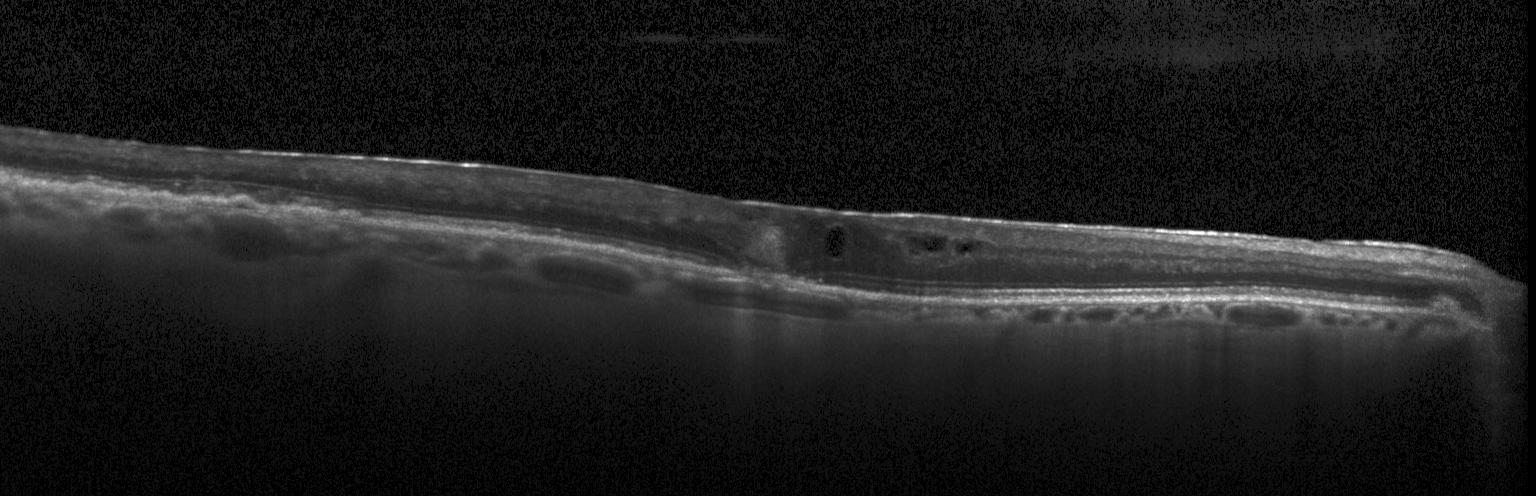 Impression: choroidal neovascularization.